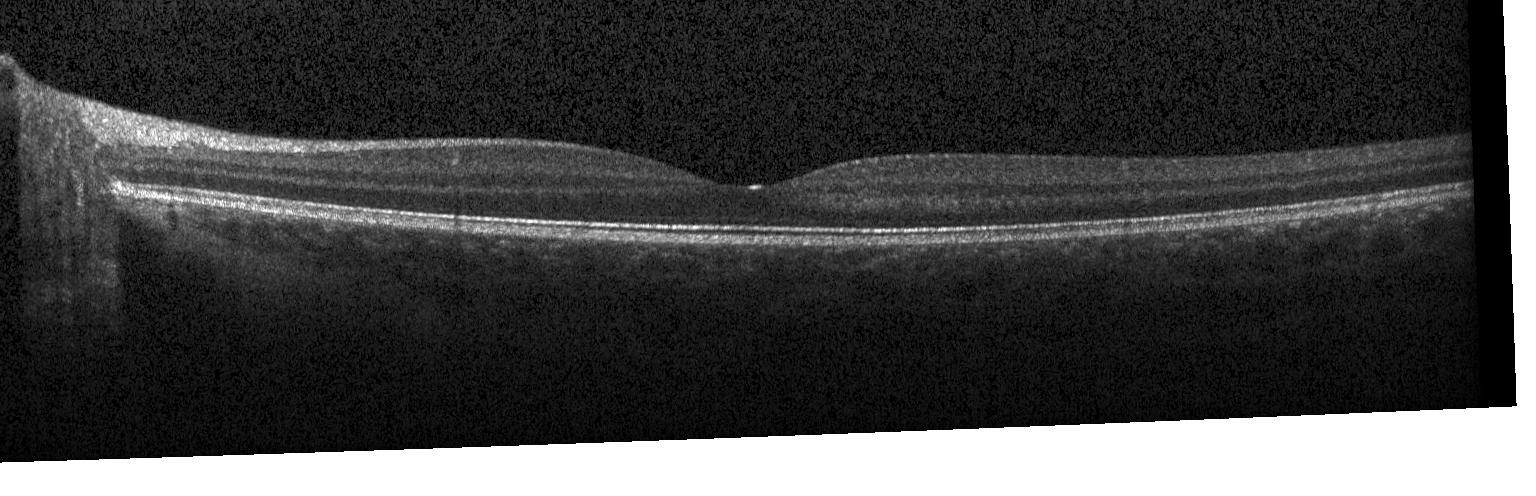
OCT finding: no CNV, DME, or drusen.